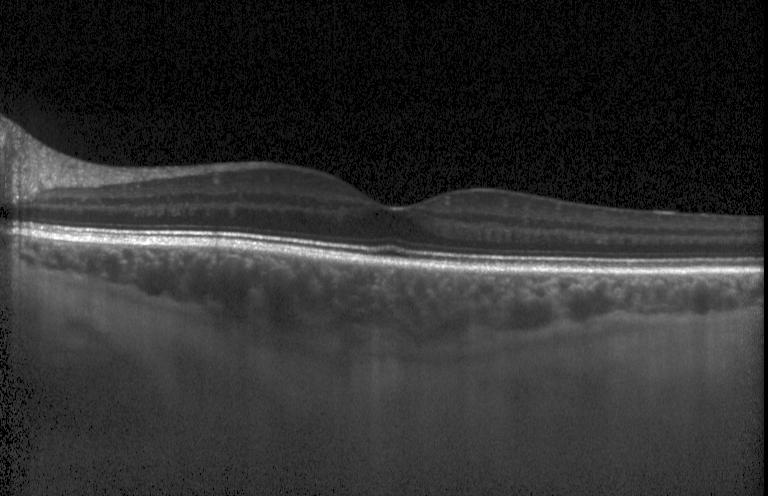
The scan shows no choroidal neovascularization, diabetic macular edema, or drusen.